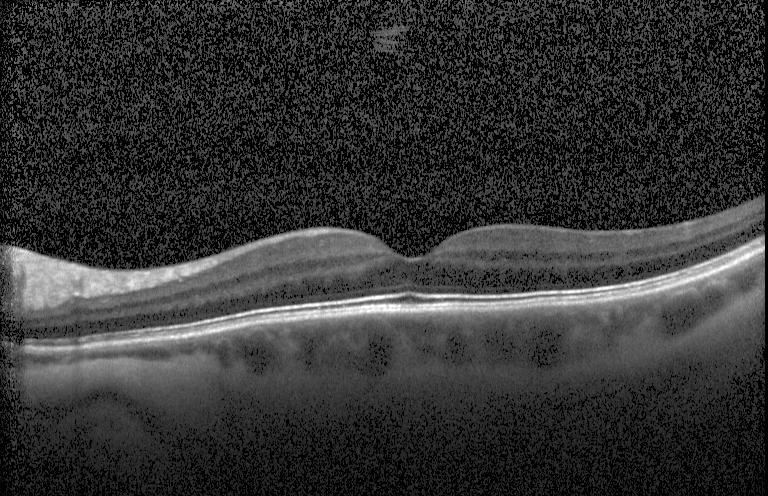
Heidelberg Spectralis · centered on the fovea · OCT line scan · spectral-domain OCT.
Assessment: no evidence of choroidal neovascularization, diabetic macular edema, or drusen.